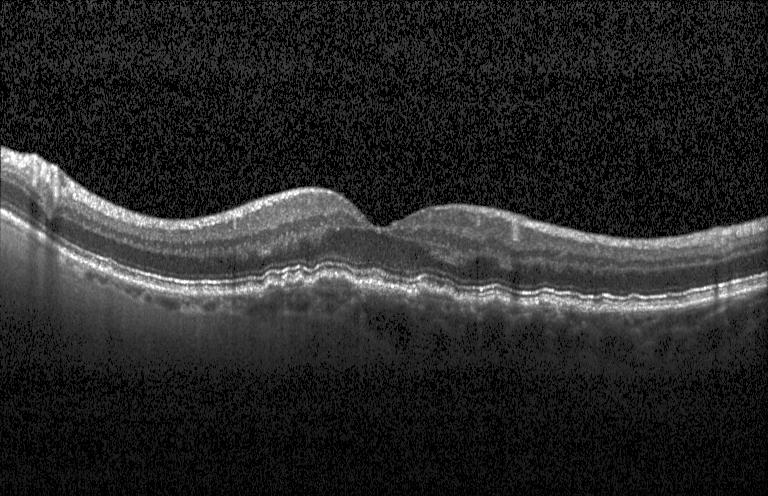
The scan shows sub-RPE drusenoid deposits.